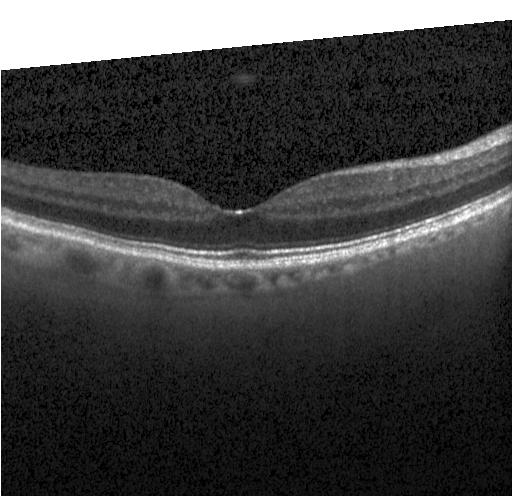
Diagnosis: neither CNV, DME, nor drusen.